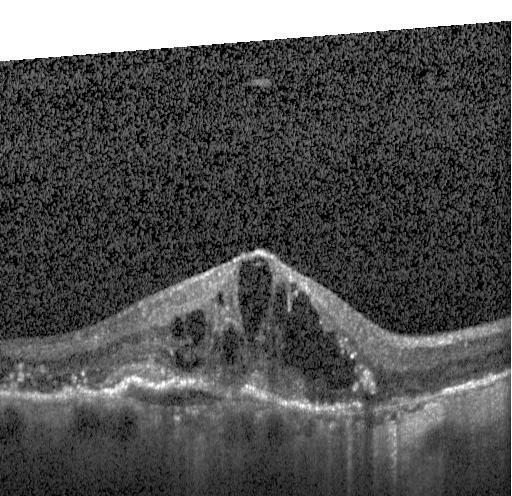 Spectral-domain optical coherence tomography; retinal OCT B-scan; Heidelberg Spectralis OCT system; fovea-centered.
Impression: a choroidal neovascular membrane.